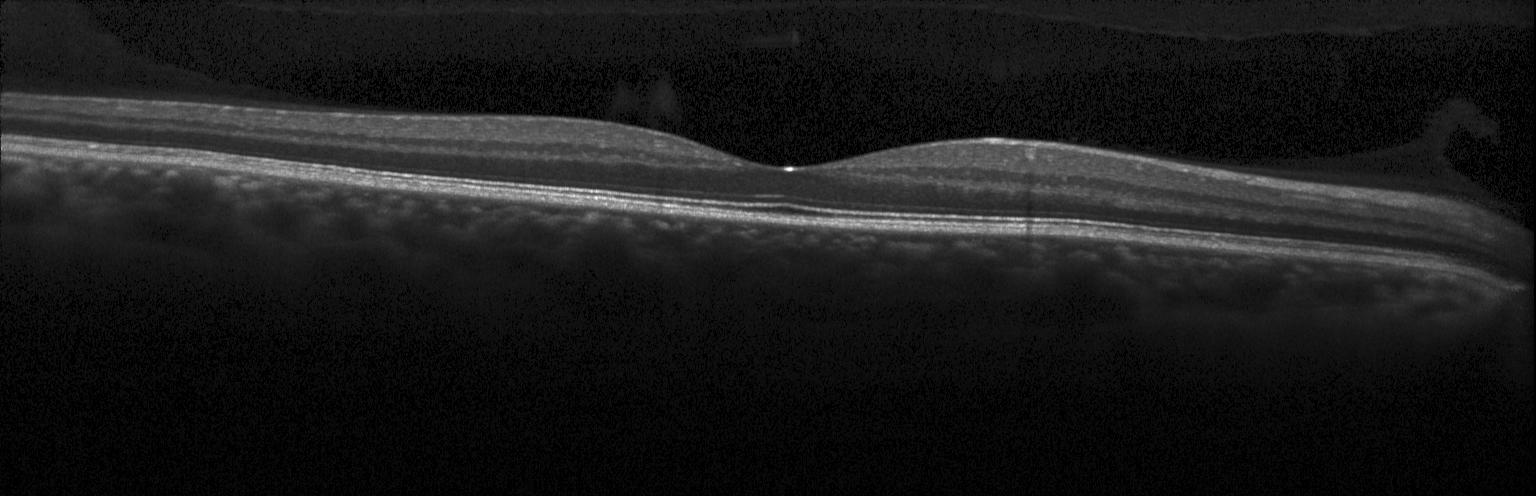

OCT finding: no evidence of CNV, DME, or drusen.